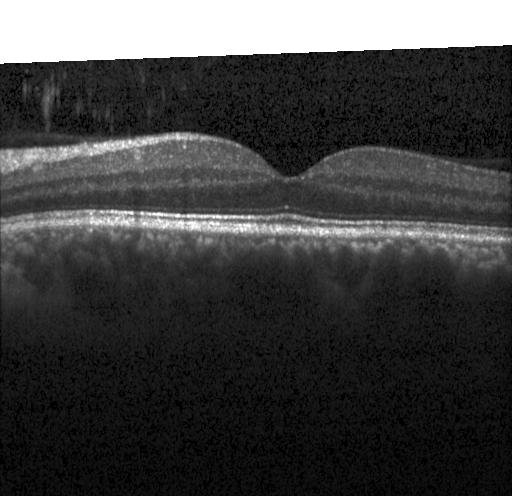 Horizontal scan through the fovea; spectral-domain optical coherence tomography; acquired on a Heidelberg Spectralis; retinal OCT cross-section — Finding: no evidence of CNV, DME, or drusen.